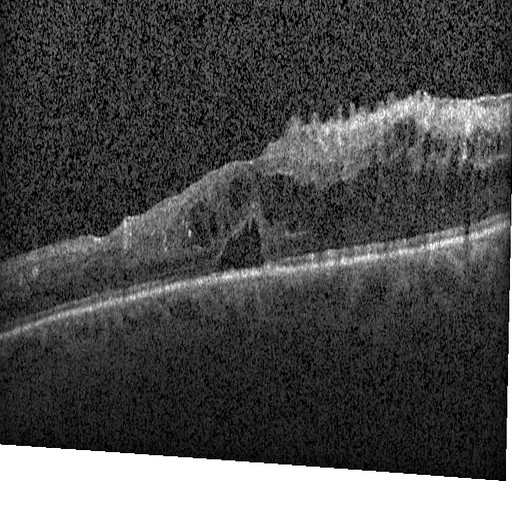
Heidelberg Spectralis · OCT line scan
Impression: diabetic macular edema (DME).